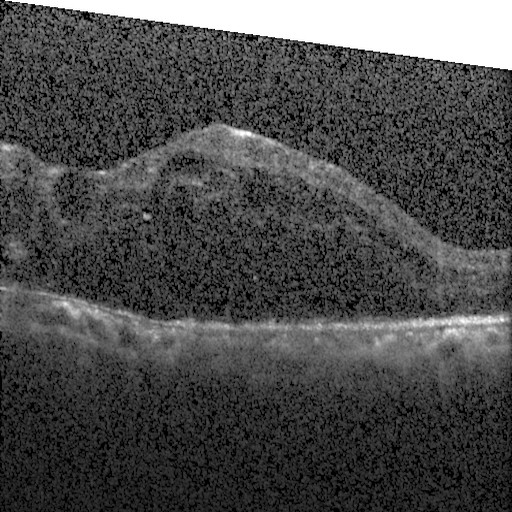
Spectral-domain OCT, horizontal scan through the fovea, acquired on a Heidelberg Spectralis, OCT line scan — Finding: diabetic macular edema.